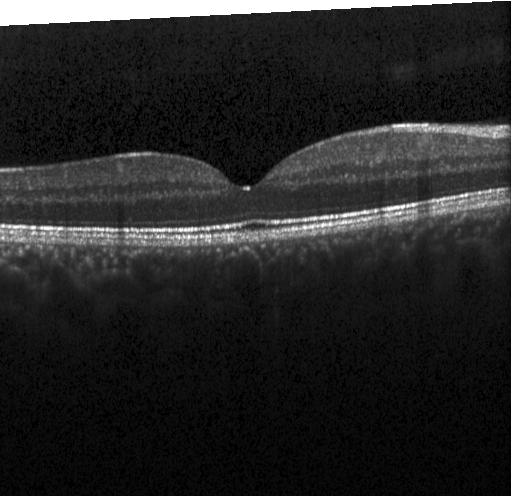 Macular scan; retinal OCT B-scan — Neither choroidal neovascularization, diabetic macular edema, nor drusen.